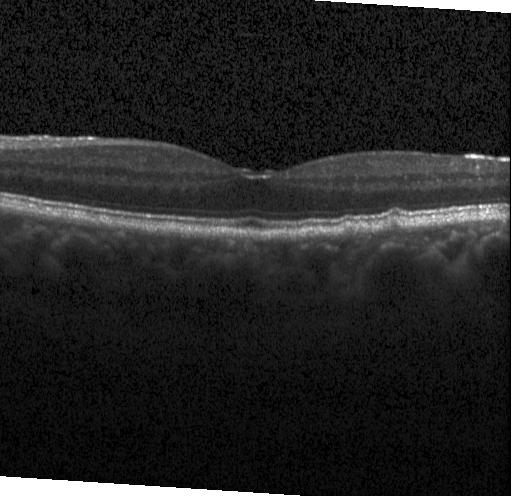
Retinal OCT B-scan · spectral-domain OCT · macular scan · acquired on a Heidelberg Spectralis
Finding: drusen.